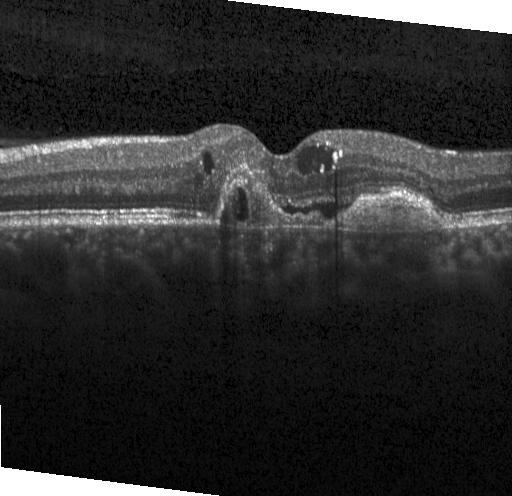 Finding: choroidal neovascularization (CNV).